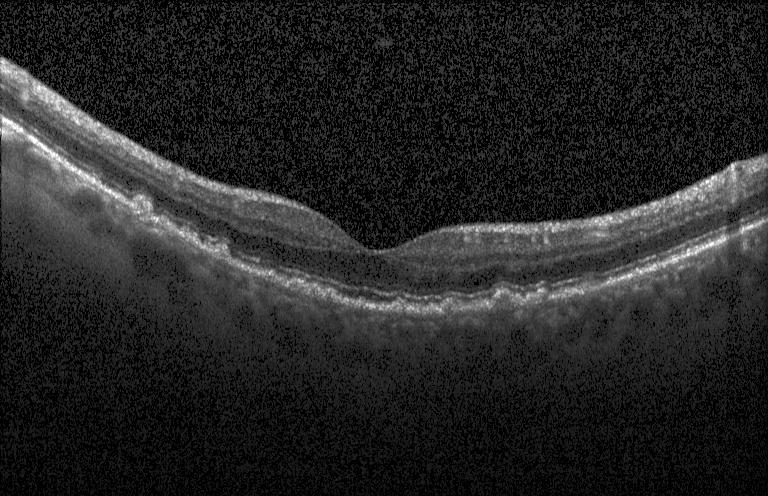

Impression: sub-RPE drusenoid deposits.